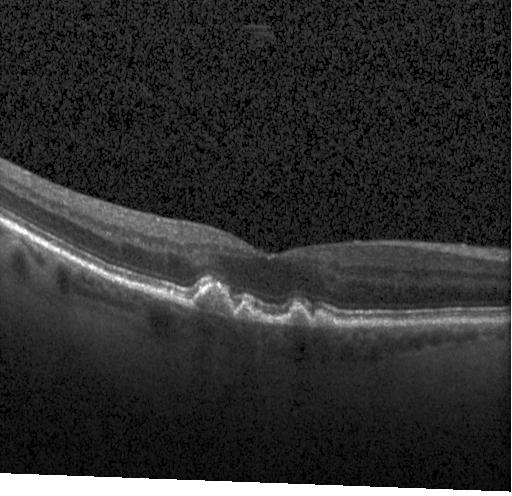 Spectral-domain OCT. Fovea-centered. Instrument: Heidelberg Spectralis. Optical coherence tomography B-scan
The scan shows multiple drusen.